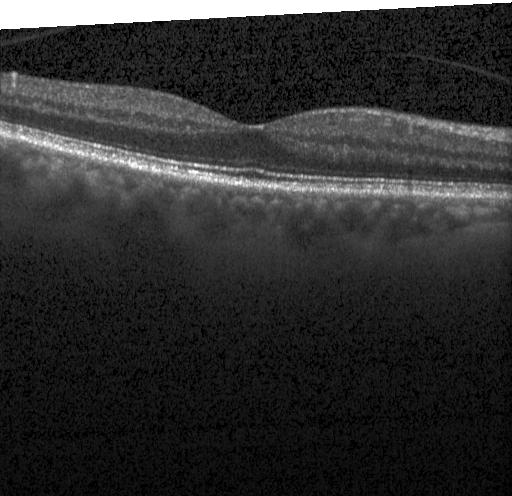
Macular OCT: neither choroidal neovascularization, diabetic macular edema, nor drusen.